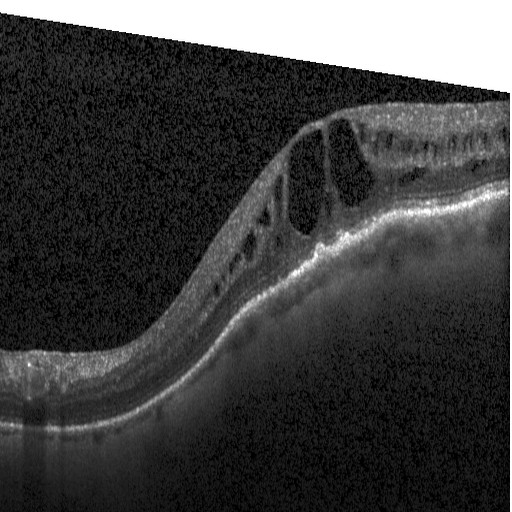

This B-scan demonstrates diabetic macular edema.